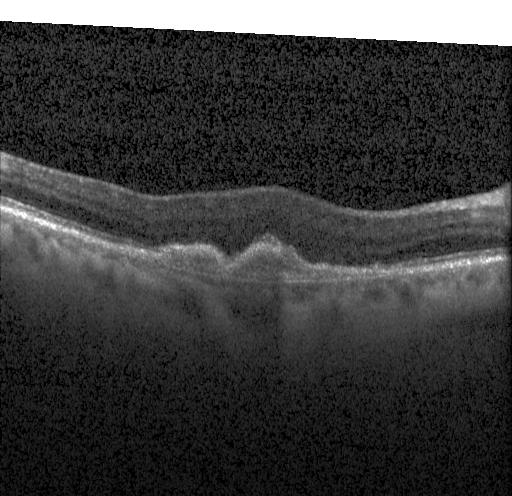 Spectral-domain OCT B-scan: choroidal neovascularization (CNV).